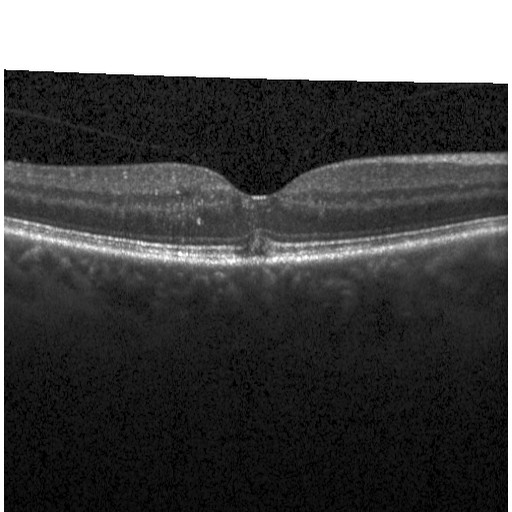

Spectral-domain optical coherence tomography. Instrument: Heidelberg Spectralis. Through the macula. Retinal OCT cross-section. Impression: DME.